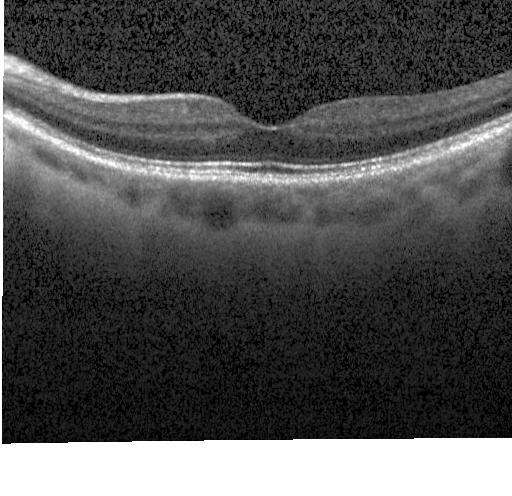
No CNV, no DME, and no drusen.